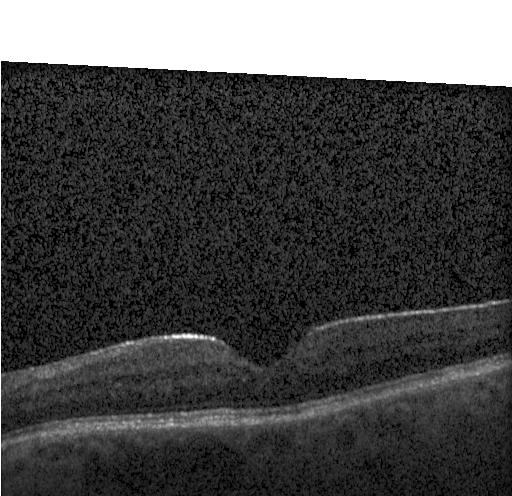
Fovea-centered. Retinal OCT B-scan.
Impression: no evidence of choroidal neovascularization, diabetic macular edema, or drusen.